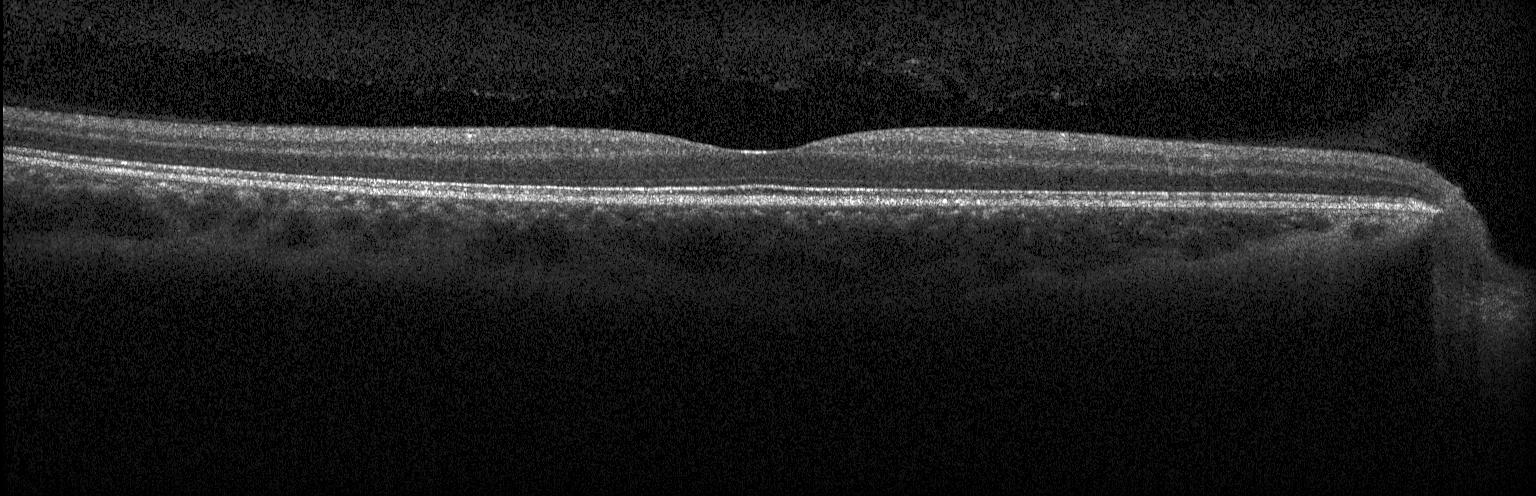 Dx: no CNV, no DME, and no drusen.